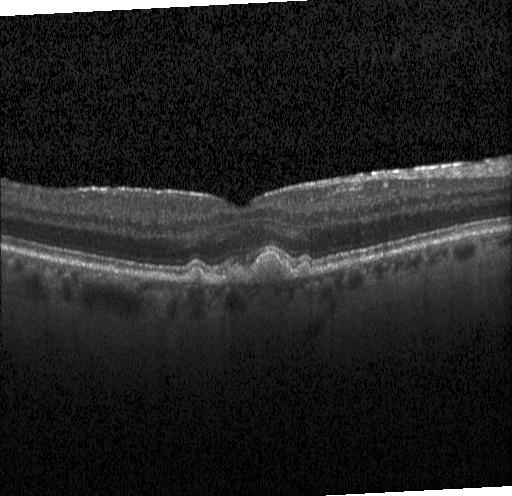

Macular OCT: drusen.